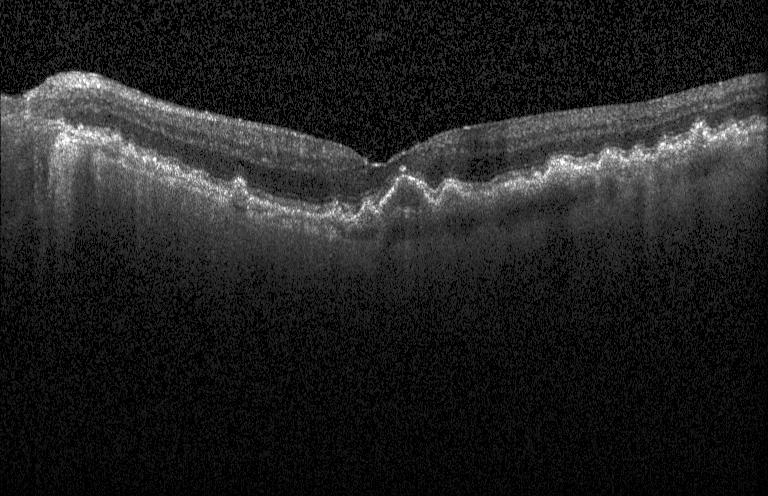

Instrument: Heidelberg Spectralis · OCT line scan — Diagnosis: drusen.